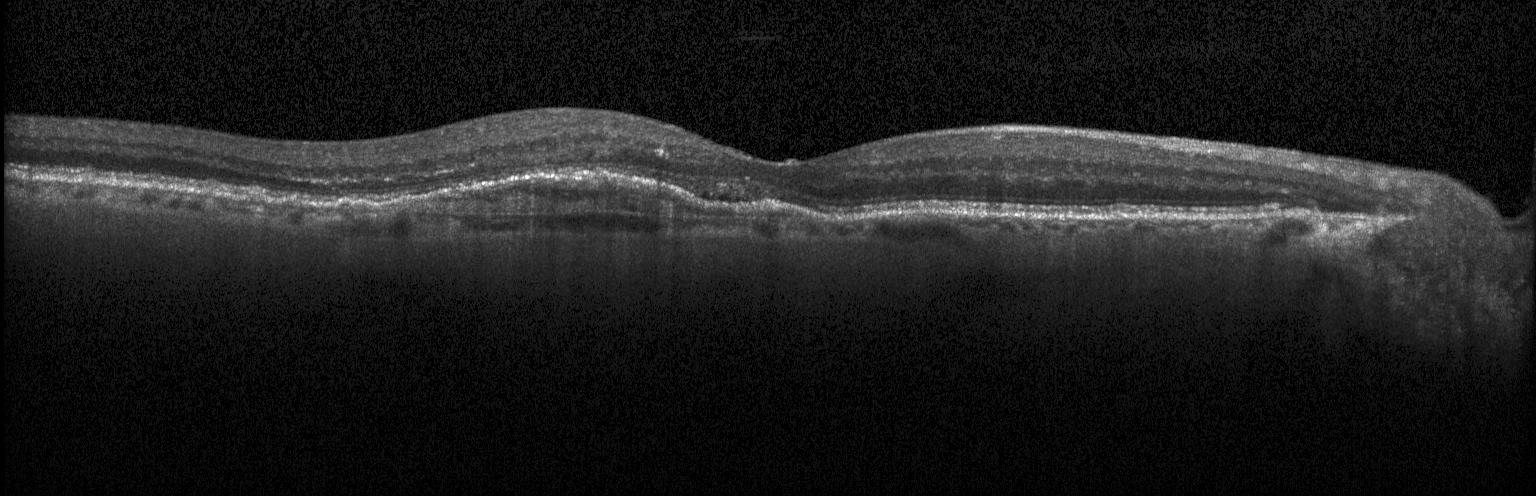

Optical coherence tomography B-scan.
The scan shows choroidal neovascularization (CNV).